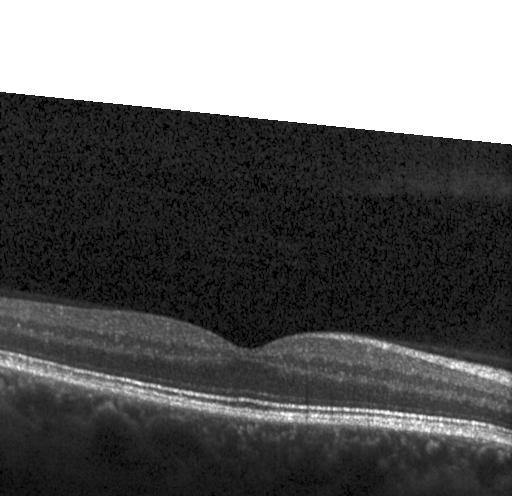 OCT finding: neither choroidal neovascularization, diabetic macular edema, nor drusen.